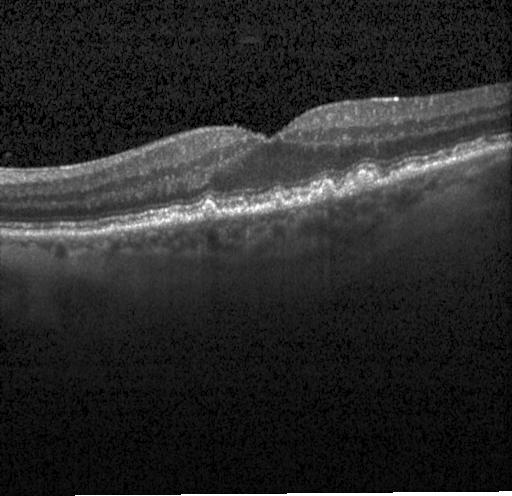 Diagnosis: multiple drusen.